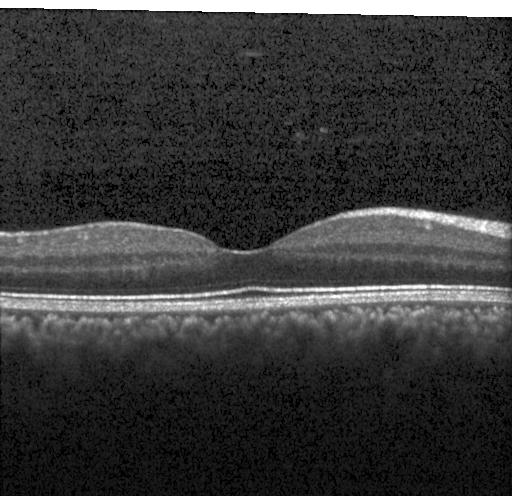 OCT B-scan; SD-OCT
Diagnosis: neither CNV, DME, nor drusen.